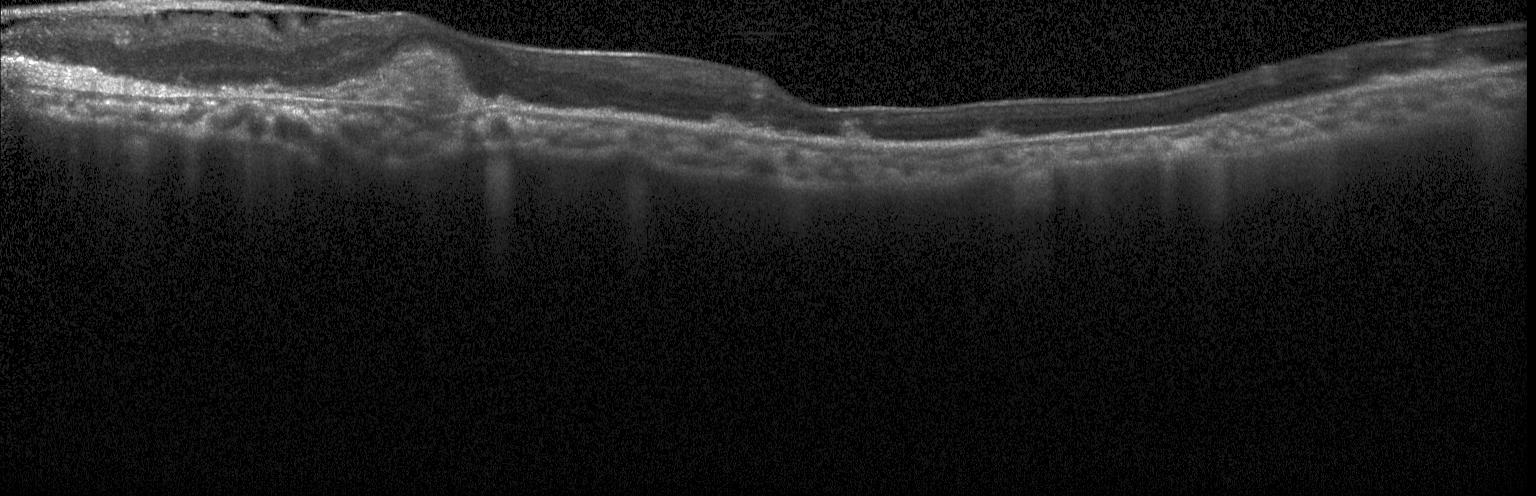 Impression: a choroidal neovascular membrane.